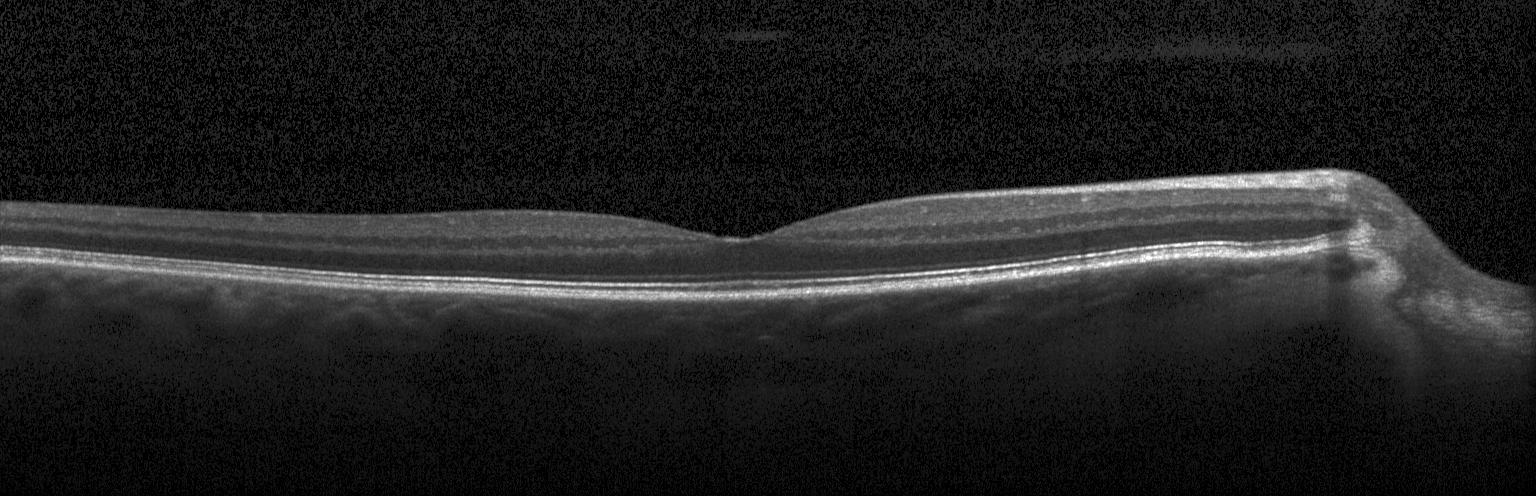 Optical coherence tomography scan — Diagnosis: neither choroidal neovascularization, diabetic macular edema, nor drusen.